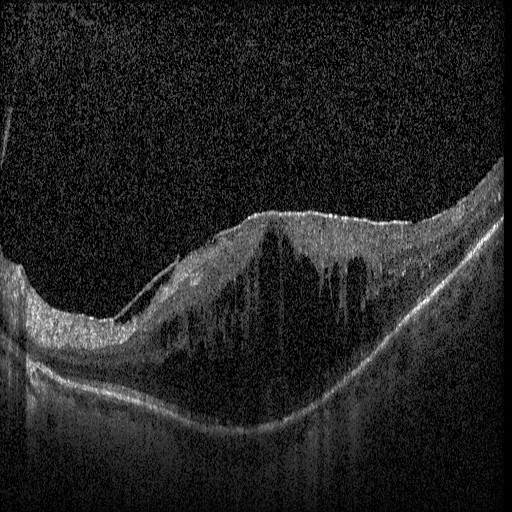

SD-OCT. Optical coherence tomography B-scan
Assessment: diabetic macular edema.